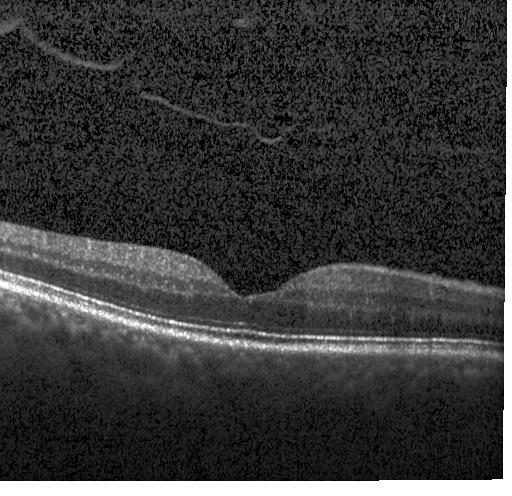 Optical coherence tomography scan. This B-scan demonstrates no choroidal neovascularization, diabetic macular edema, or drusen.